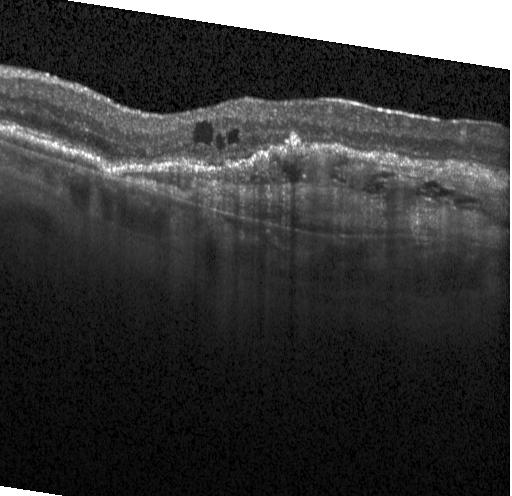
OCT finding: choroidal neovascularization (CNV).